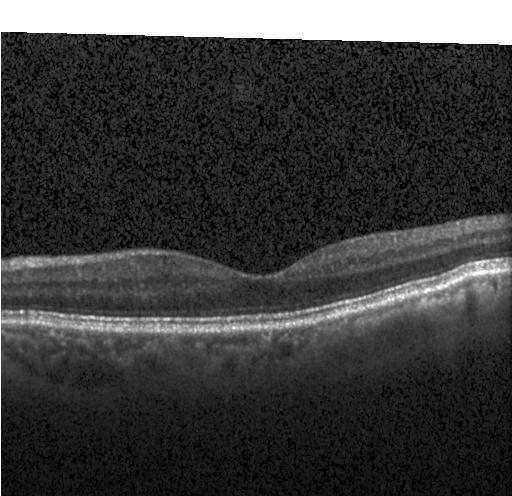 OCT B-scan showing neither choroidal neovascularization, diabetic macular edema, nor drusen.